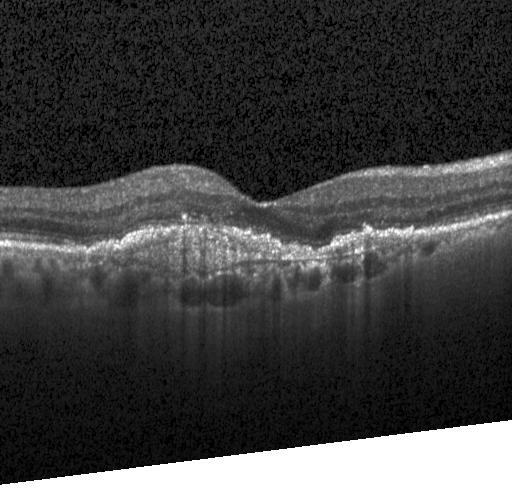
Diagnosis: a choroidal neovascular membrane.